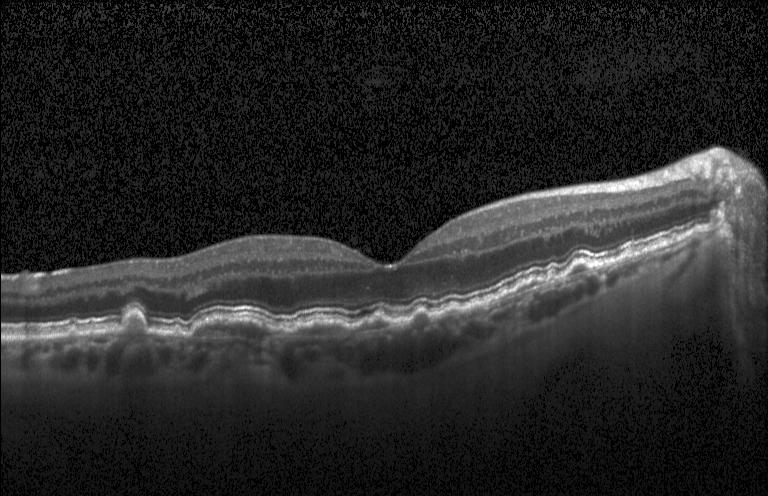

Fovea-centered · optical coherence tomography B-scan · spectral-domain OCT.
Impression: drusen.